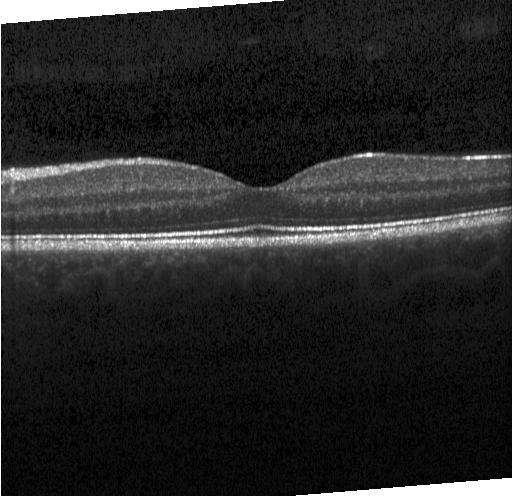
Assessment: neither choroidal neovascularization, diabetic macular edema, nor drusen.